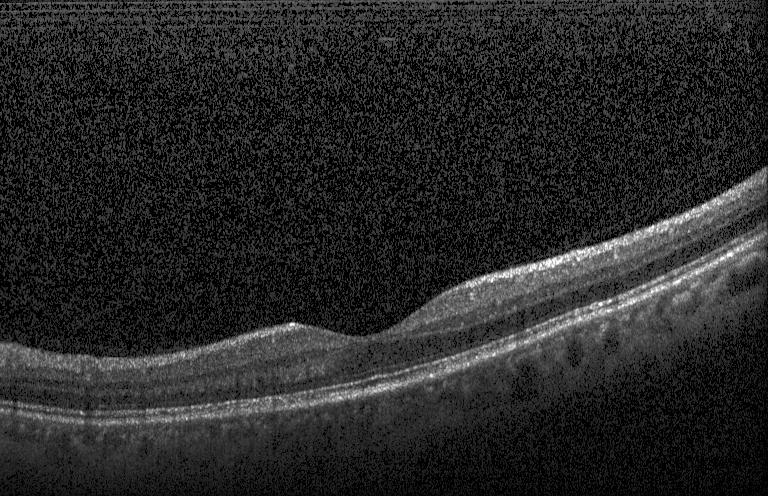

Optical coherence tomography scan. Impression: no choroidal neovascularization, diabetic macular edema, or drusen.